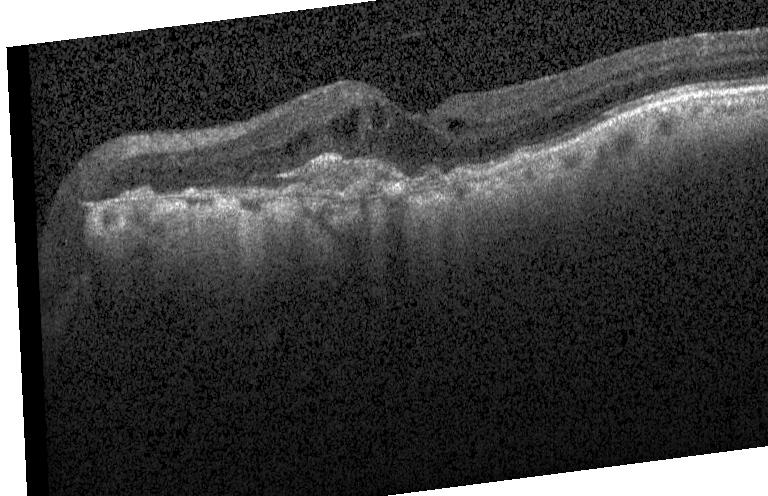
OCT B-scan · acquired on a Heidelberg Spectralis.
A choroidal neovascular membrane.